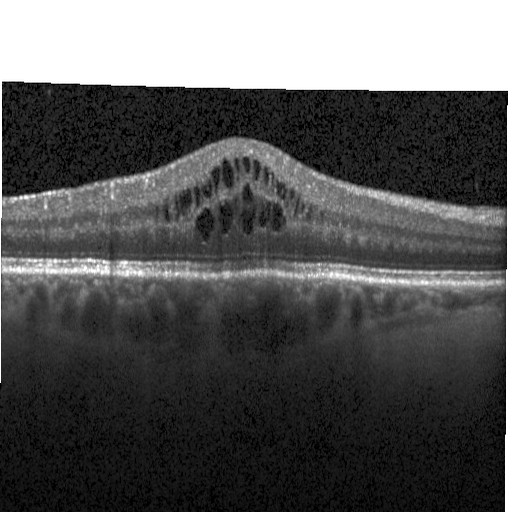
Diagnosis: diabetic macular edema (DME).